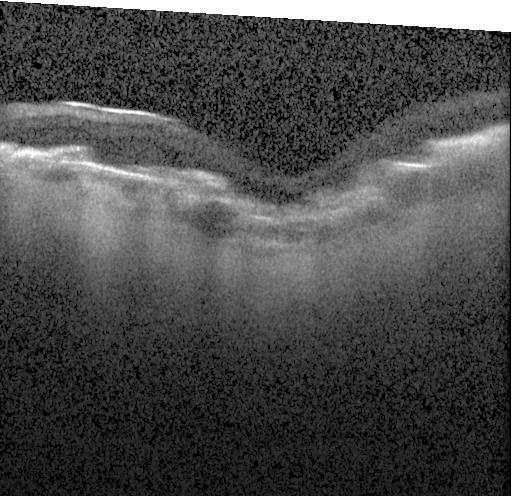 Retinal OCT B-scan.
The scan shows CNV.